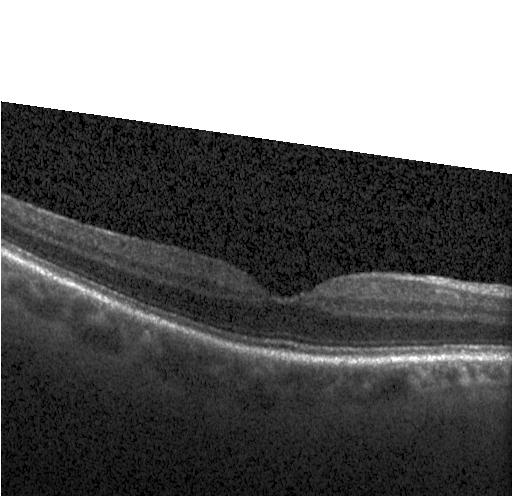 OCT B-scan; SD-OCT; instrument: Heidelberg Spectralis
This B-scan demonstrates no CNV, DME, or drusen.